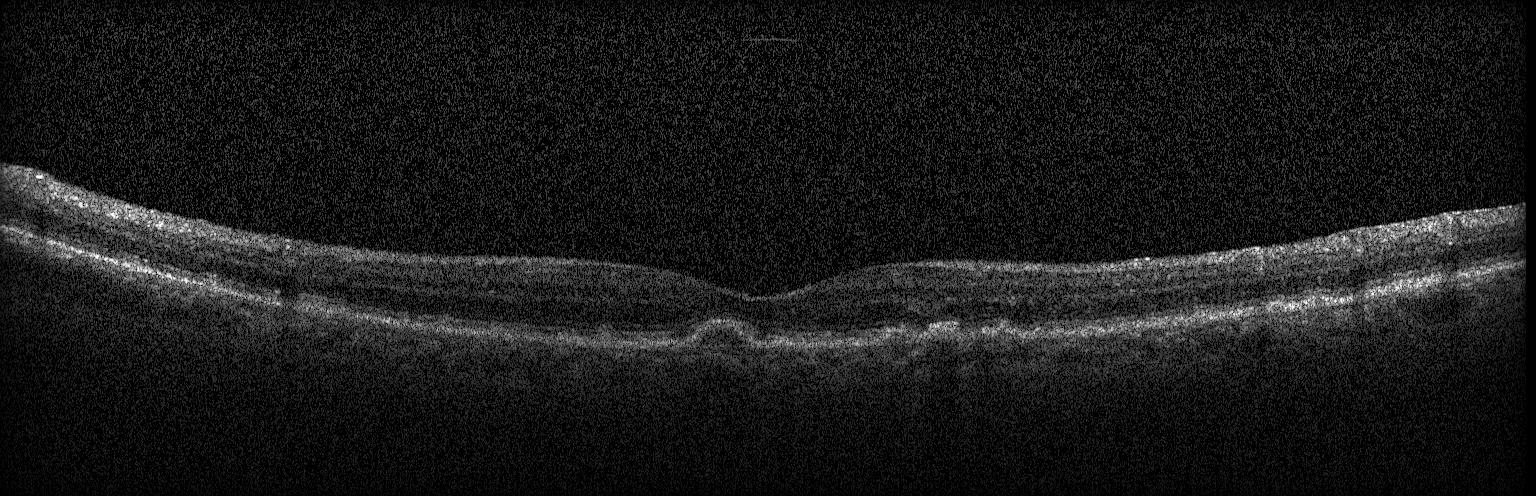 Heidelberg Spectralis OCT system, macular scan, retinal OCT B-scan, spectral-domain optical coherence tomography — Diagnosis: multiple drusen.